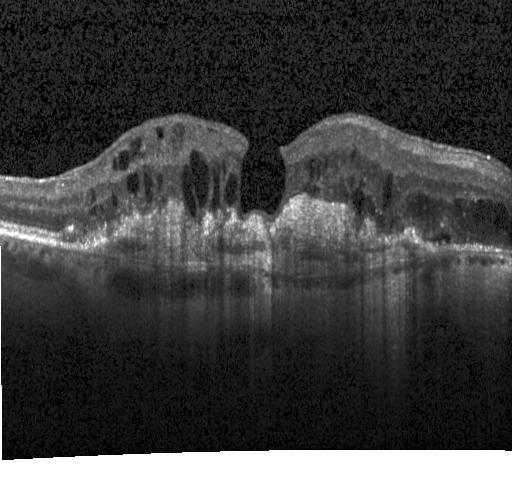

Optical coherence tomography B-scan. Acquired on a Heidelberg Spectralis. SD-OCT. Horizontal scan through the fovea — Dx: a choroidal neovascular membrane.